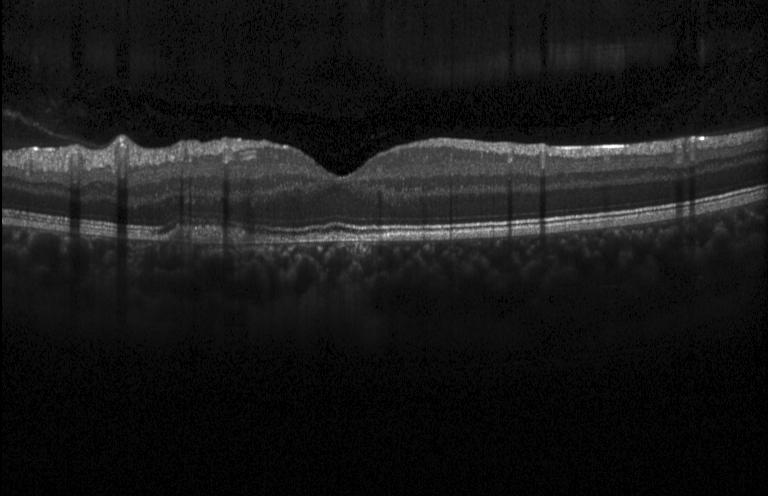
Spectral-domain optical coherence tomography, OCT line scan, macular scan
Dx: multiple drusen.